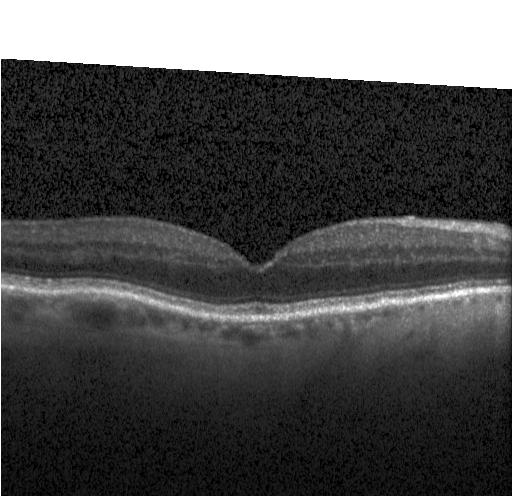 Optical coherence tomography B-scan. Heidelberg Spectralis
Finding: no choroidal neovascularization, diabetic macular edema, or drusen.